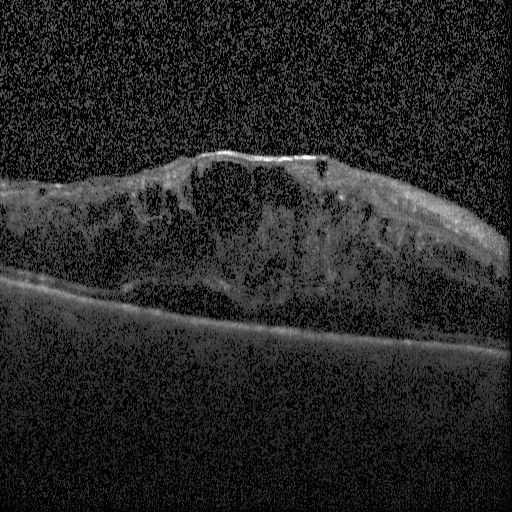 OCT line scan
Finding: DME.